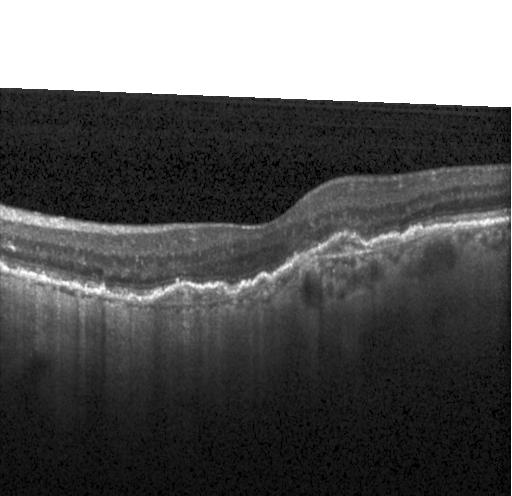 Assessment: a choroidal neovascular membrane.